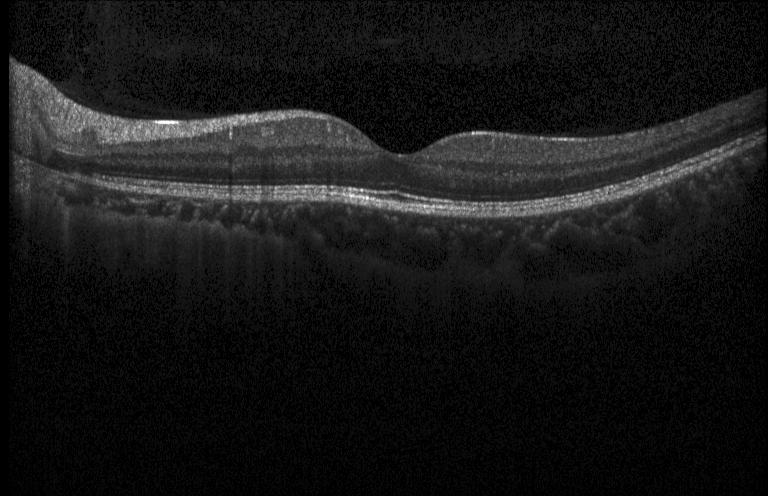 Acquired on a Heidelberg Spectralis, horizontal scan through the fovea, OCT B-scan. Impression: neither choroidal neovascularization, diabetic macular edema, nor drusen.